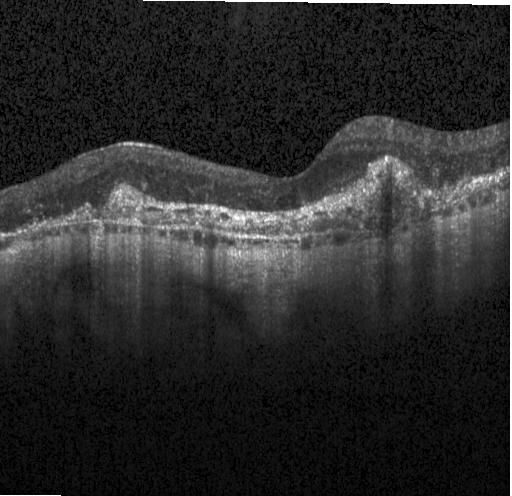
Diagnosis: choroidal neovascularization.